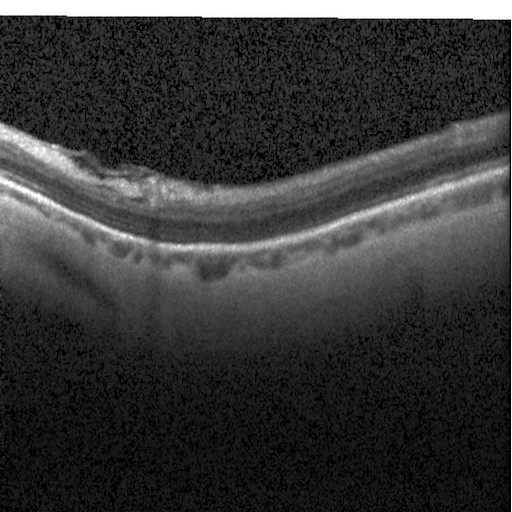 Finding: diabetic macular edema (DME).